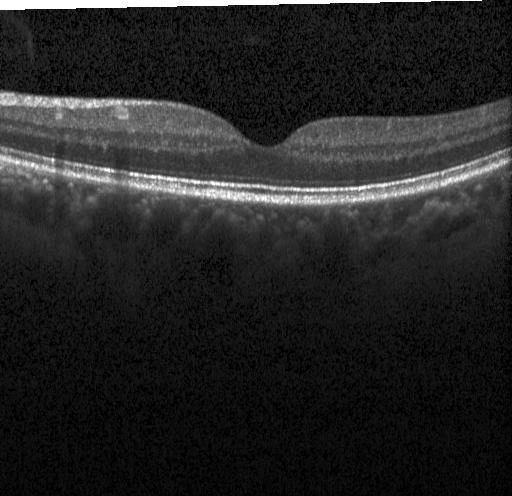

This B-scan demonstrates neither choroidal neovascularization, diabetic macular edema, nor drusen.